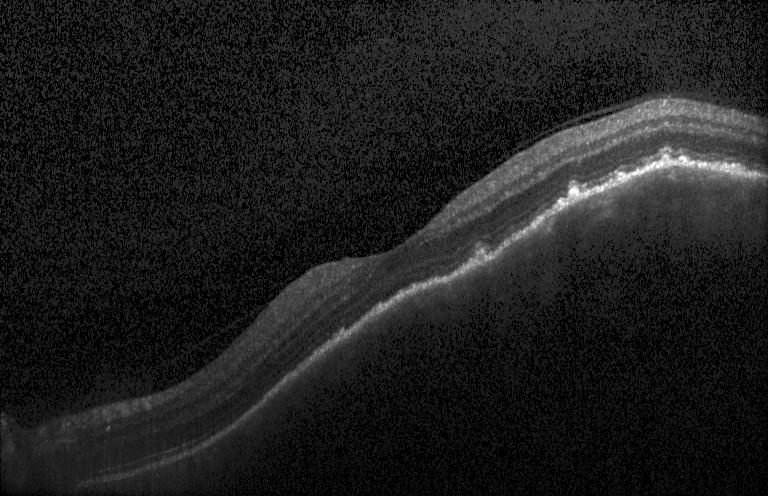 SD-OCT; fovea-centered; acquired on a Heidelberg Spectralis; OCT B-scan. Diagnosis: drusen.